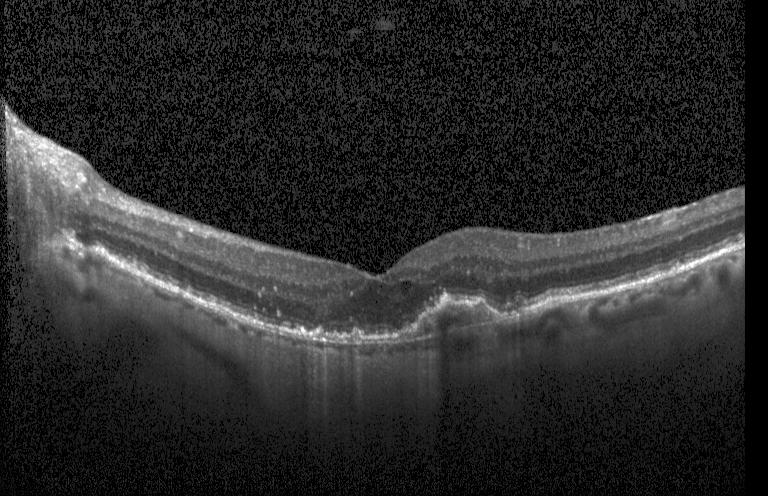
Spectral-domain OCT. Retinal OCT cross-section. Heidelberg Spectralis OCT system. Macular scan — Impression: choroidal neovascularization.